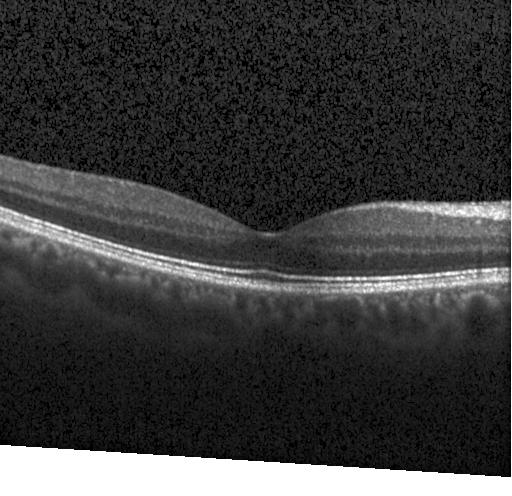

Retinal OCT B-scan. Heidelberg Spectralis OCT system
This B-scan demonstrates no choroidal neovascularization, diabetic macular edema, or drusen.